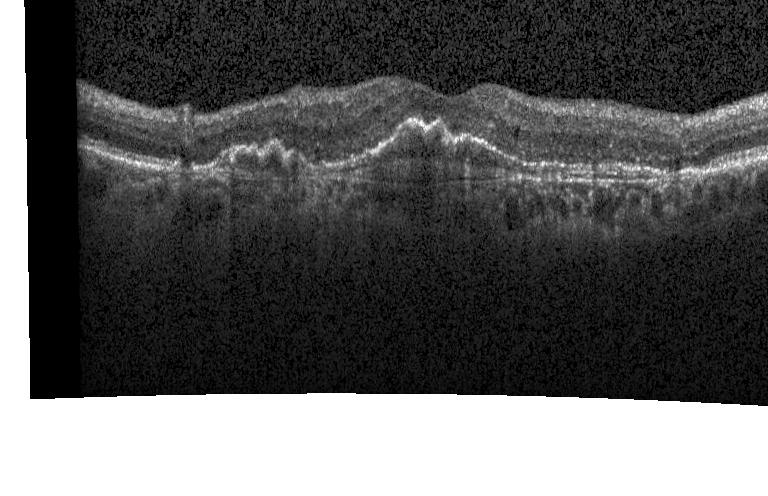
The scan shows a choroidal neovascular membrane.